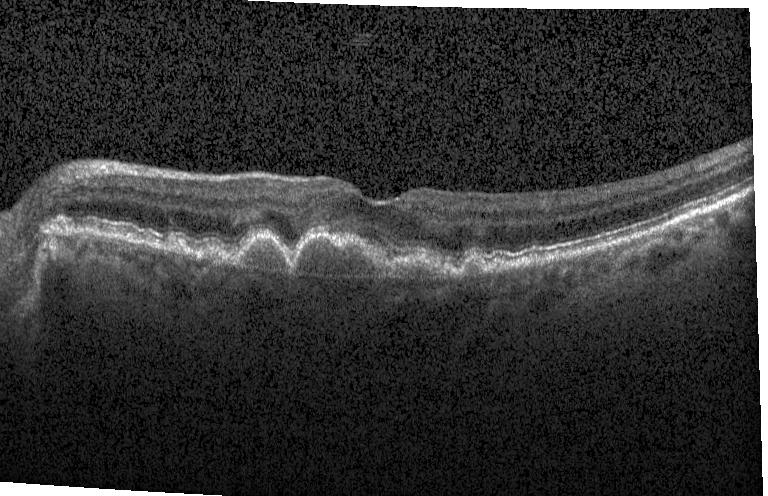
Fovea-centered. SD-OCT. Heidelberg Spectralis. Optical coherence tomography scan
The scan shows a choroidal neovascular membrane.